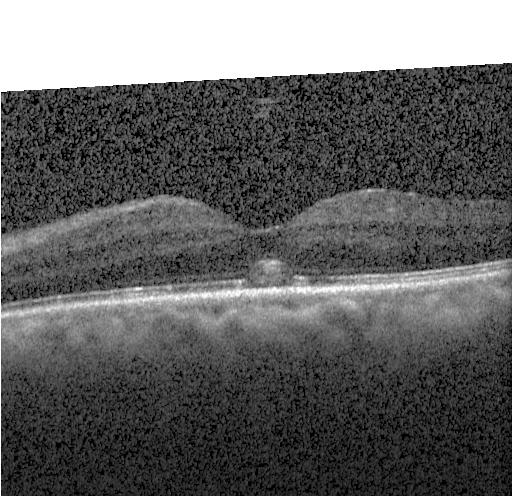
CNV.